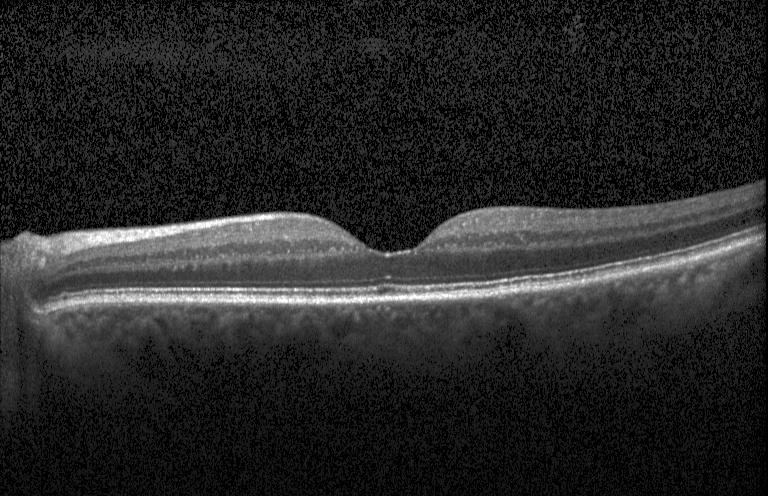
Neither CNV, DME, nor drusen.